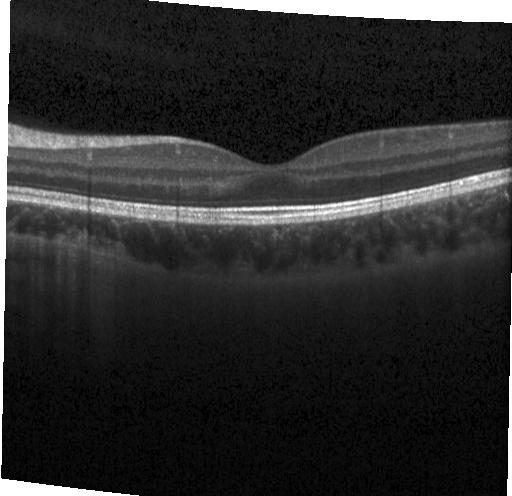 The scan shows neither choroidal neovascularization, diabetic macular edema, nor drusen.